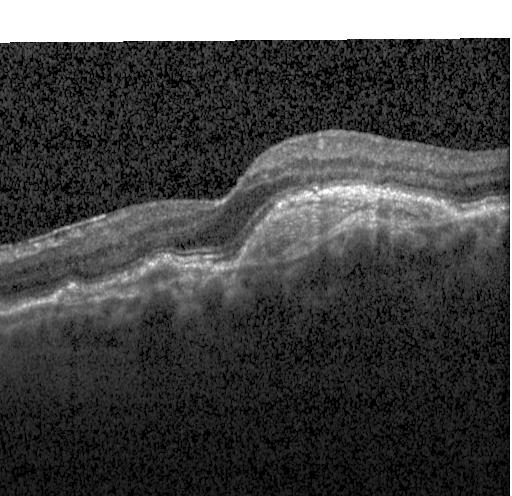 Spectral-domain OCT; centered on the fovea; Heidelberg Spectralis; optical coherence tomography scan
Impression: choroidal neovascularization (CNV).